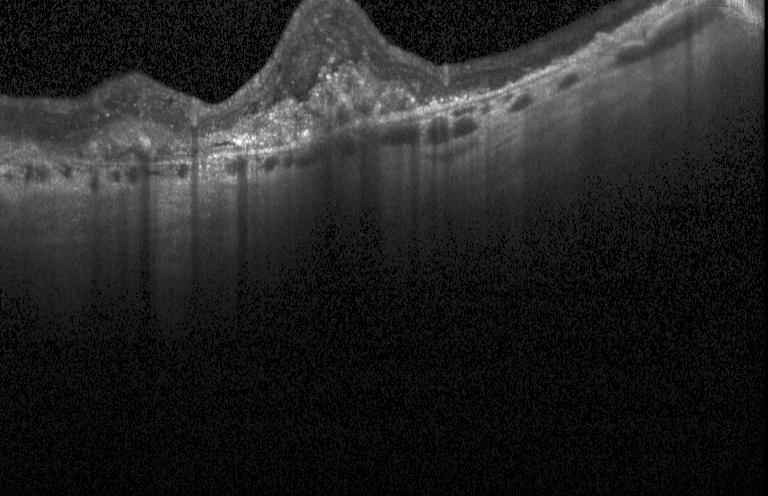 Optical coherence tomography scan. Diagnosis: CNV.